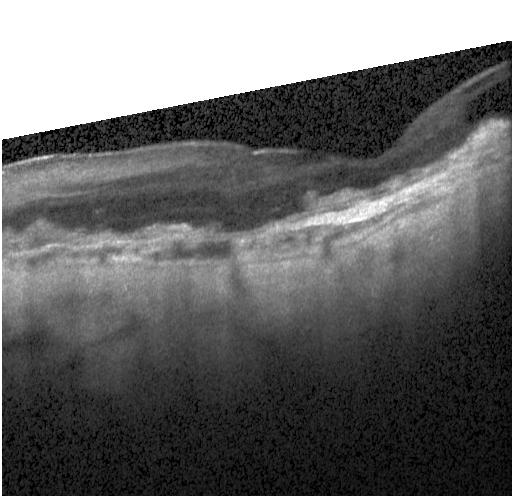

Dx: CNV.